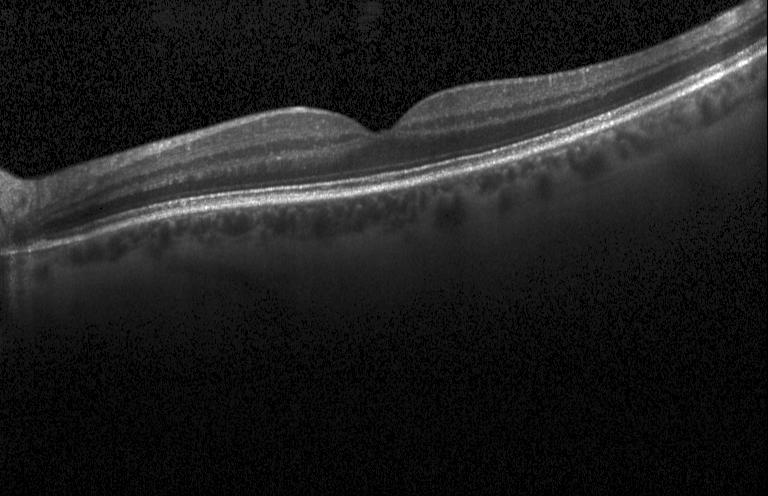

OCT finding: no evidence of choroidal neovascularization, diabetic macular edema, or drusen.